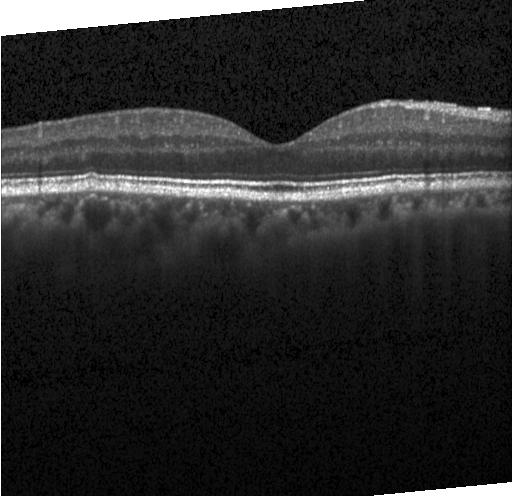

OCT line scan. The scan shows sub-RPE drusenoid deposits.